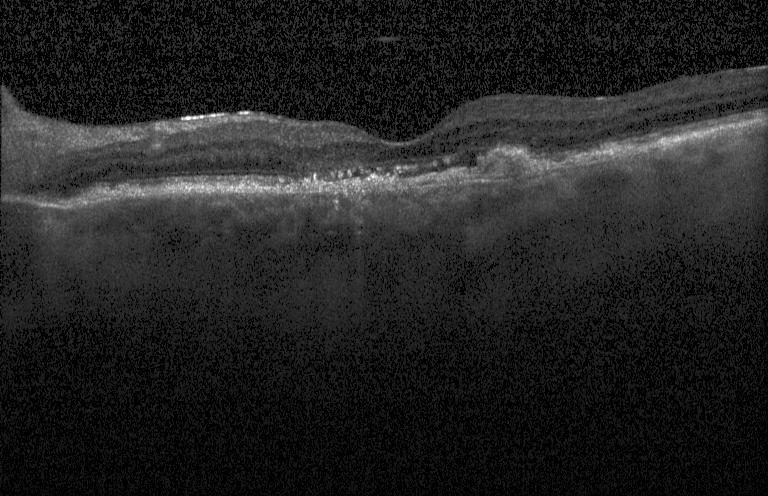

OCT line scan · Heidelberg Spectralis OCT system · SD-OCT — CNV.